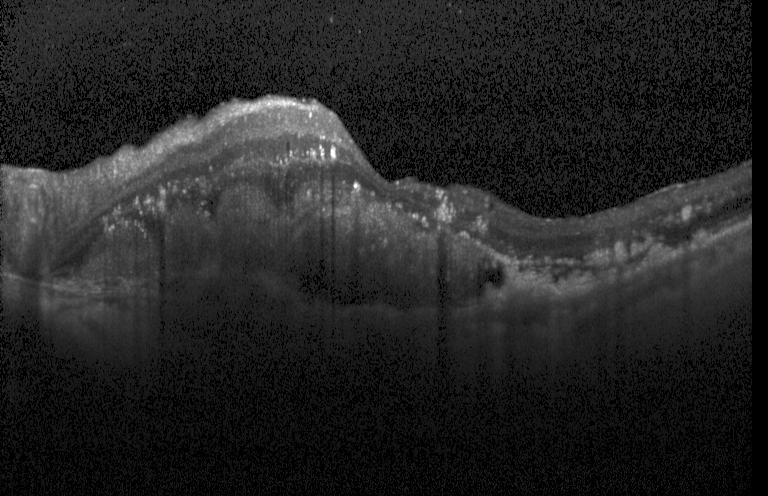 Spectral-domain OCT · OCT line scan · fovea-centered. Finding: a choroidal neovascular membrane.